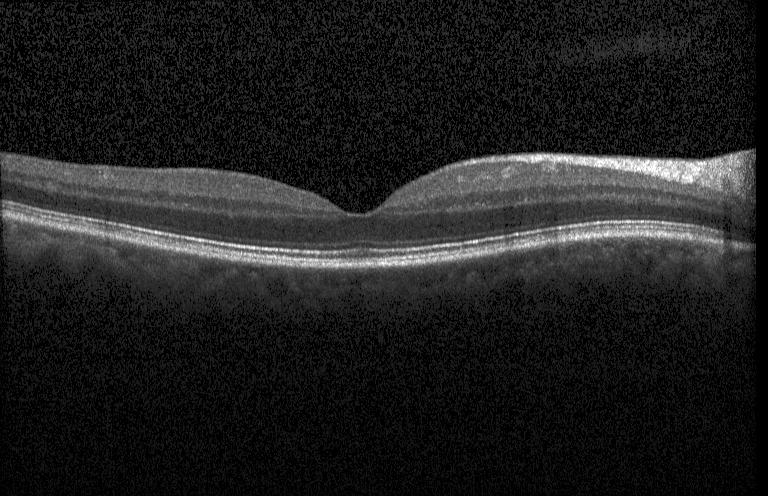 OCT finding: no CNV, DME, or drusen.